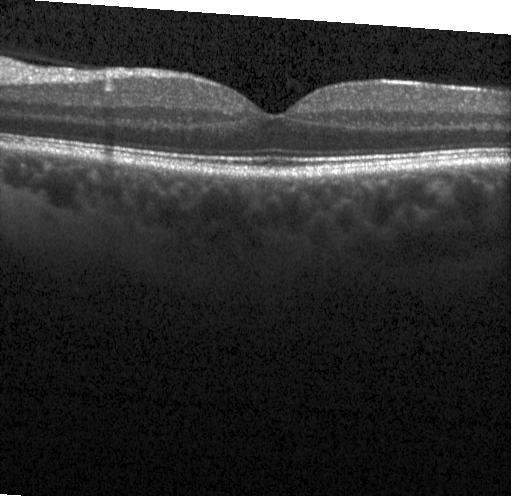 Dx: no choroidal neovascularization, diabetic macular edema, or drusen.